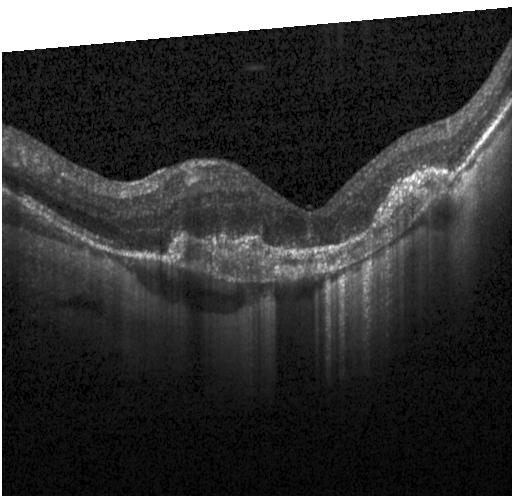
Centered on the fovea · OCT line scan · Heidelberg Spectralis OCT system. OCT finding: a choroidal neovascular membrane.